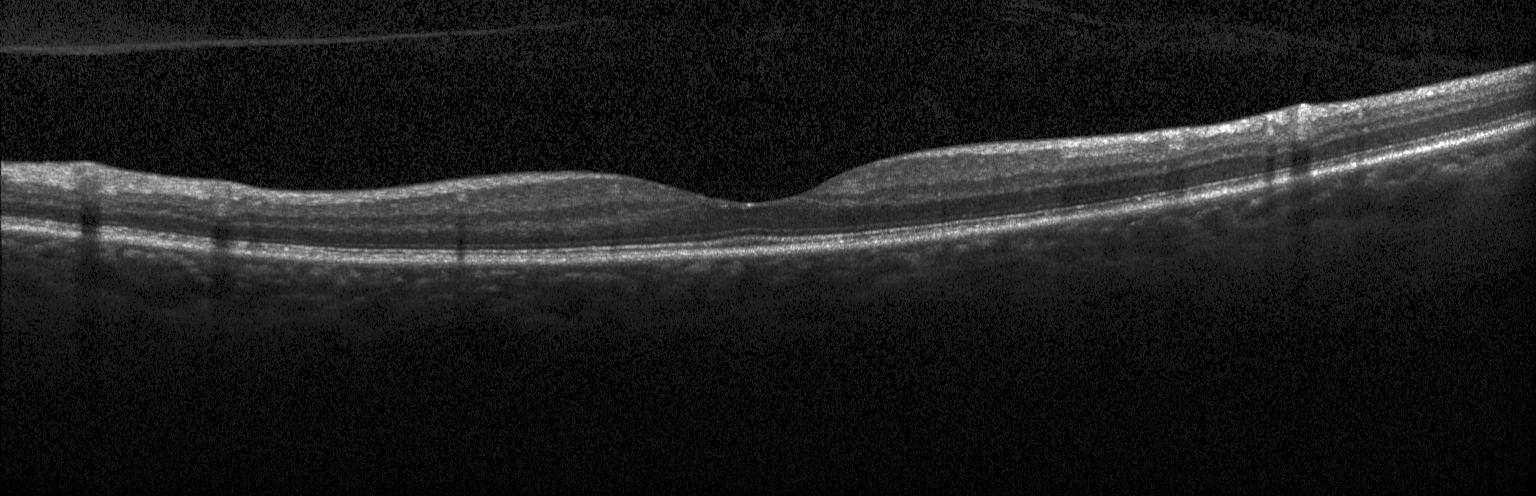 Retinal OCT cross-section
Assessment: no evidence of CNV, DME, or drusen.